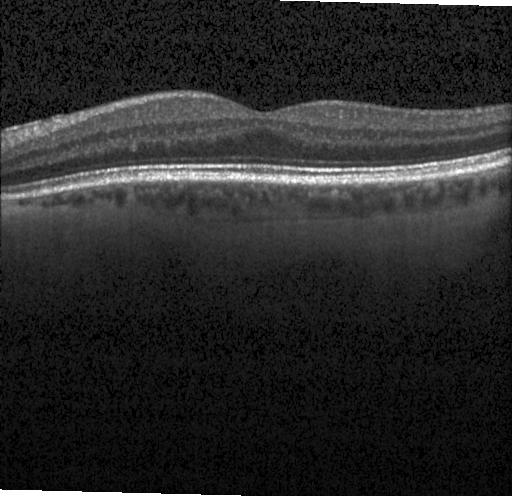
This B-scan demonstrates no CNV, DME, or drusen.